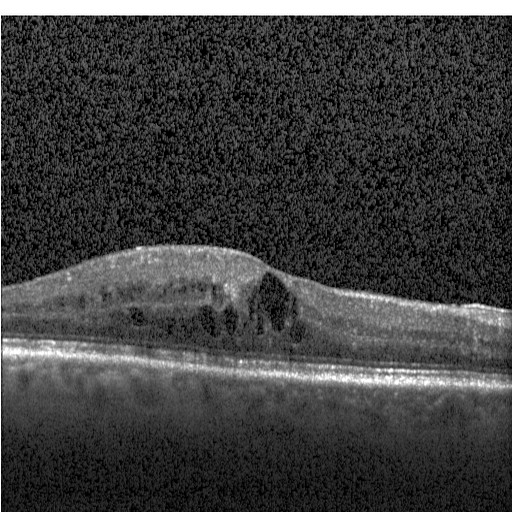

OCT finding: diabetic macular edema (DME).